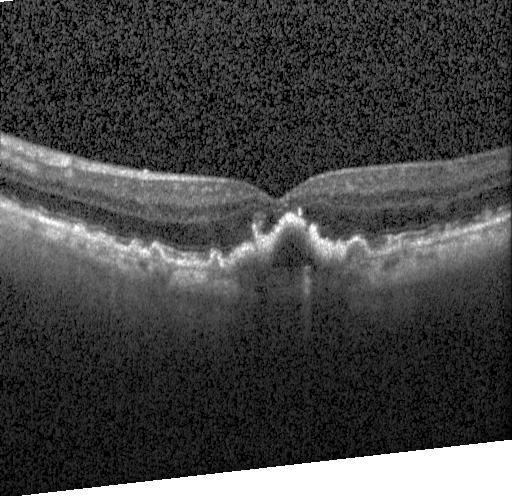 Acquired on a Heidelberg Spectralis, optical coherence tomography scan, through the macula.
Finding: CNV.